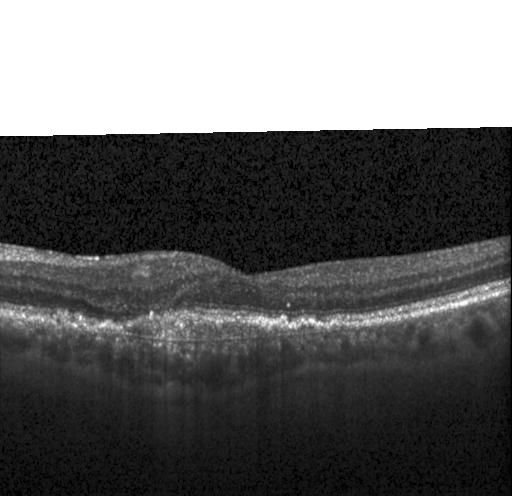

Heidelberg Spectralis OCT system; OCT line scan; SD-OCT; macular scan — Dx: a choroidal neovascular membrane.